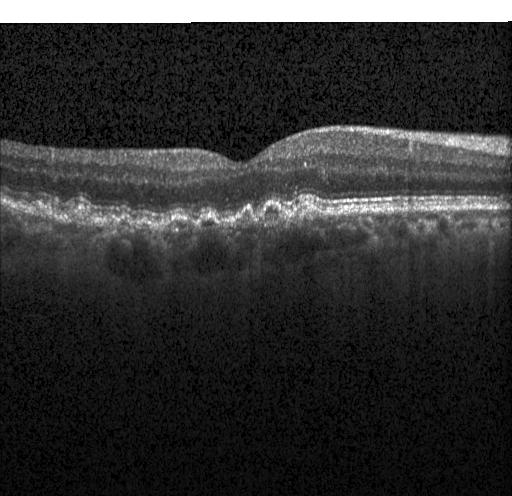
Diagnosis: sub-RPE drusenoid deposits.